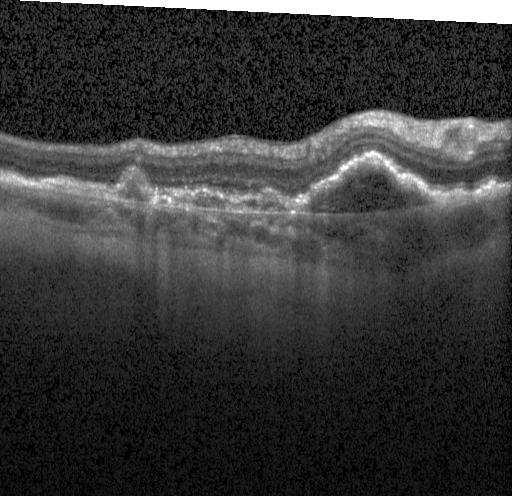
SD-OCT; retinal OCT B-scan; Heidelberg Spectralis OCT system — This B-scan demonstrates choroidal neovascularization (CNV).